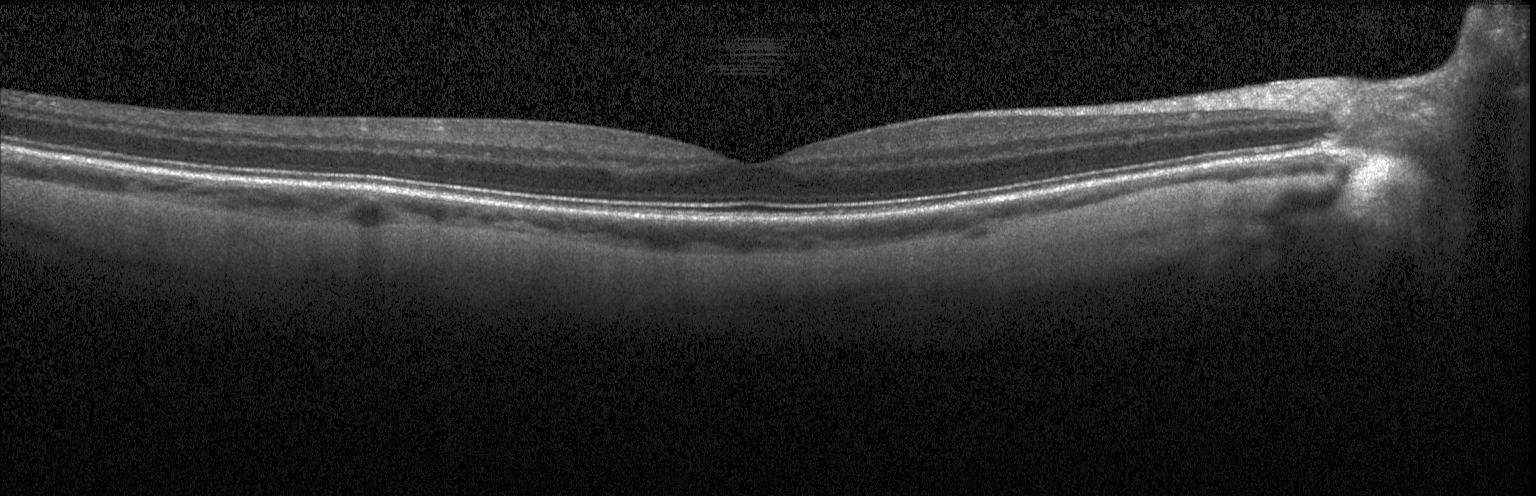
Optical coherence tomography scan; Heidelberg Spectralis OCT system. Impression: no evidence of choroidal neovascularization, diabetic macular edema, or drusen.